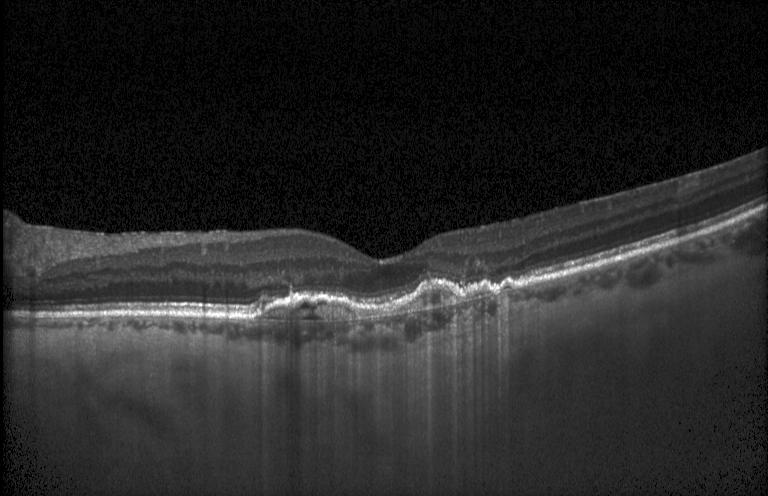
OCT finding: a choroidal neovascular membrane.